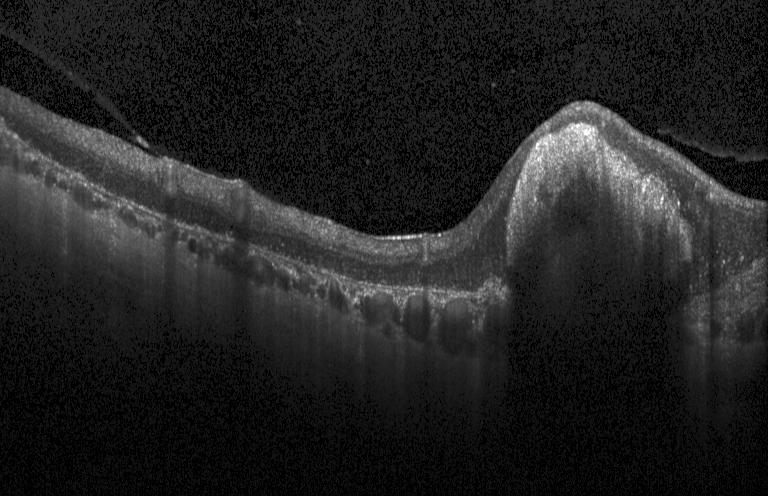
Finding: a choroidal neovascular membrane.